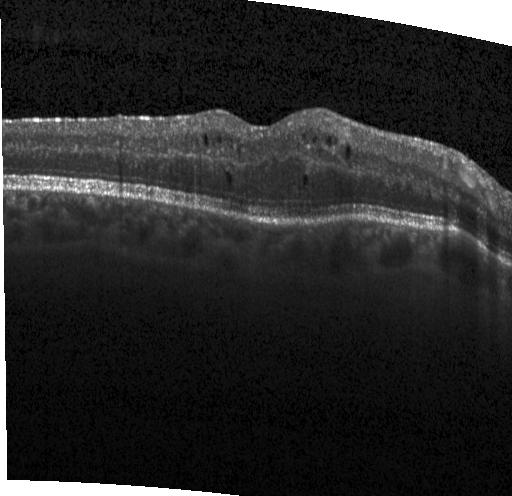 Retinal OCT B-scan
Diabetic macular edema (DME).